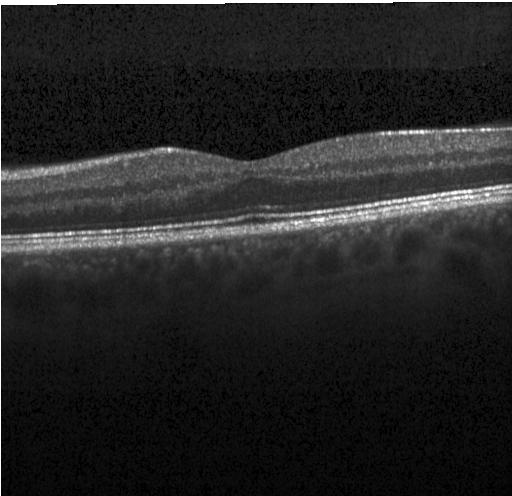

Finding: no choroidal neovascularization, diabetic macular edema, or drusen.